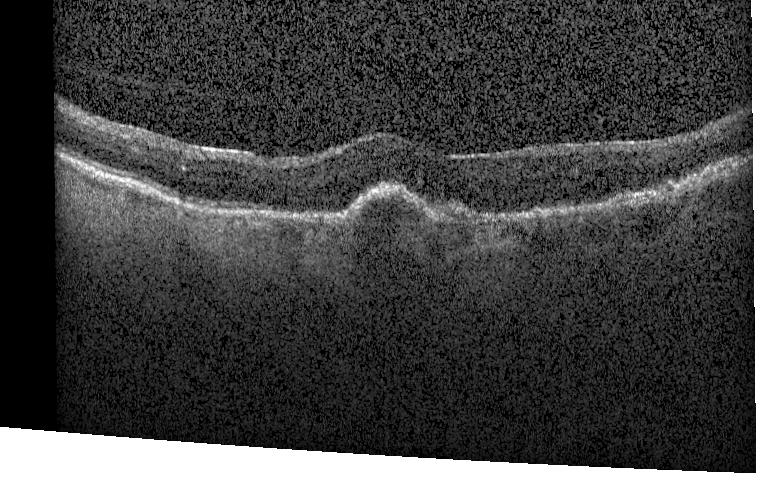
Macular scan. Spectral-domain optical coherence tomography. Retinal OCT cross-section. Heidelberg Spectralis.
OCT finding: a choroidal neovascular membrane.